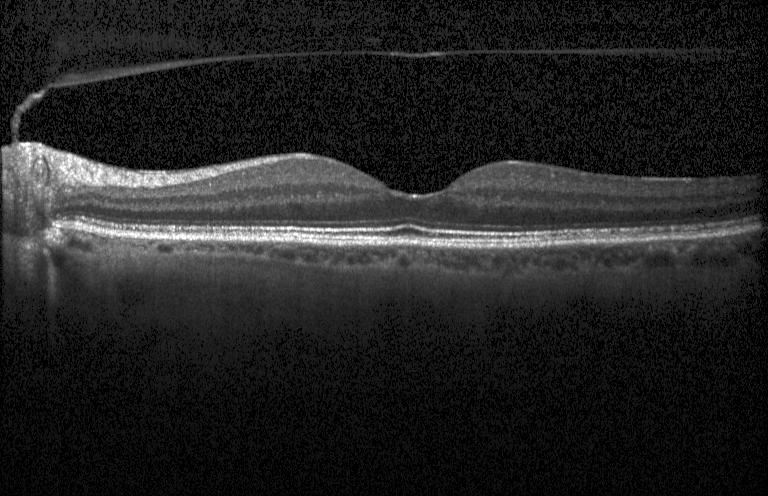 Optical coherence tomography B-scan · acquired on a Heidelberg Spectralis
Assessment: no choroidal neovascularization, no diabetic macular edema, and no drusen.